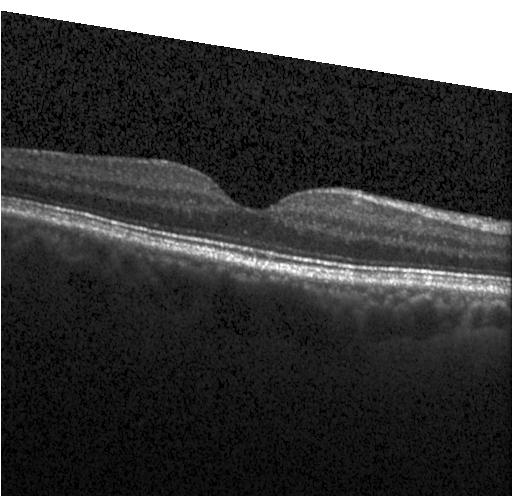 Finding: neither choroidal neovascularization, diabetic macular edema, nor drusen.